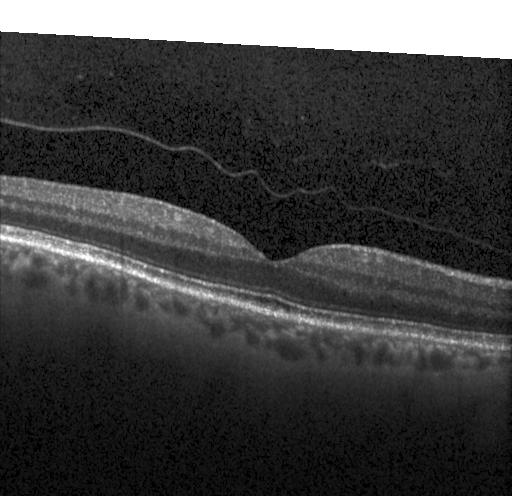

Spectral-domain OCT B-scan: neither choroidal neovascularization, diabetic macular edema, nor drusen.